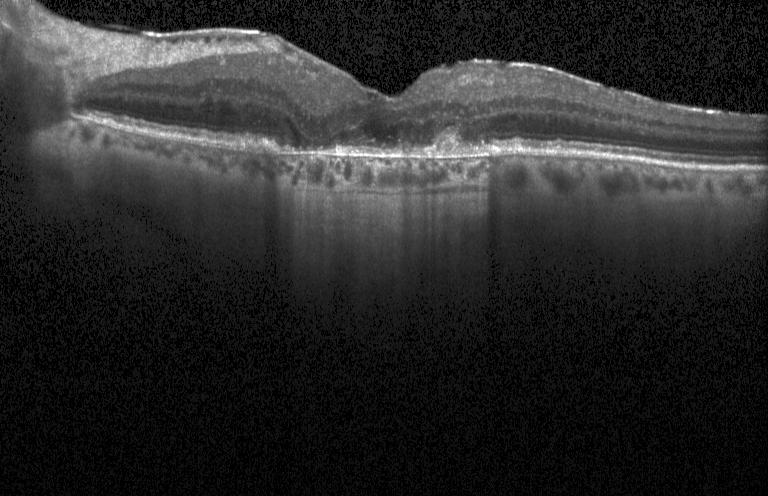
Retinal OCT cross-section. SD-OCT — Assessment: choroidal neovascularization (CNV).